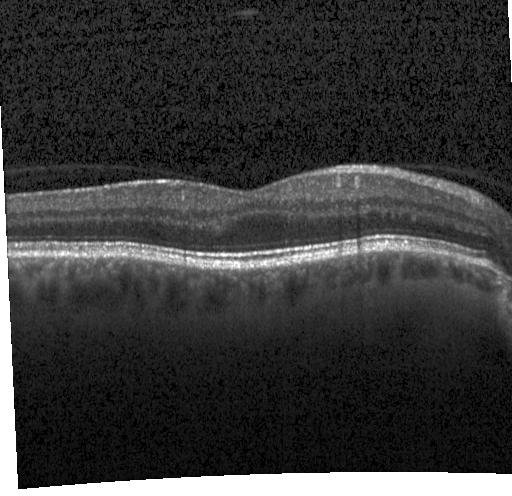
Retinal OCT B-scan, Heidelberg Spectralis.
The scan shows no CNV, DME, or drusen.